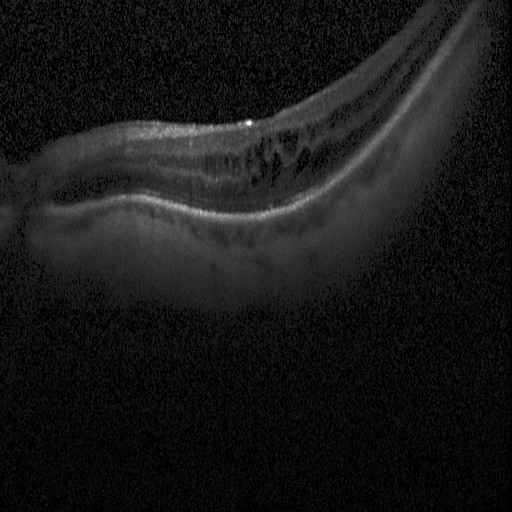

OCT B-scan.
Finding: diabetic macular edema.